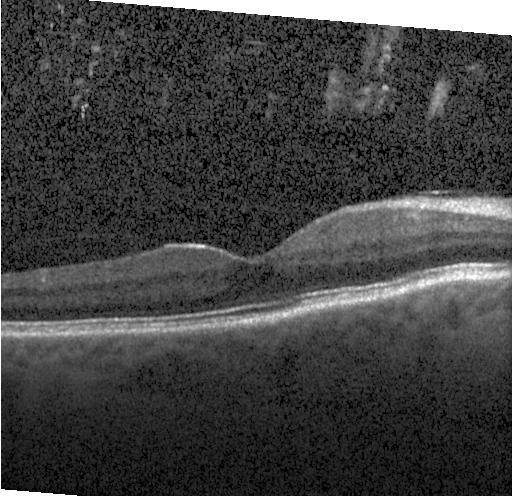

Impression: no choroidal neovascularization, no diabetic macular edema, and no drusen.